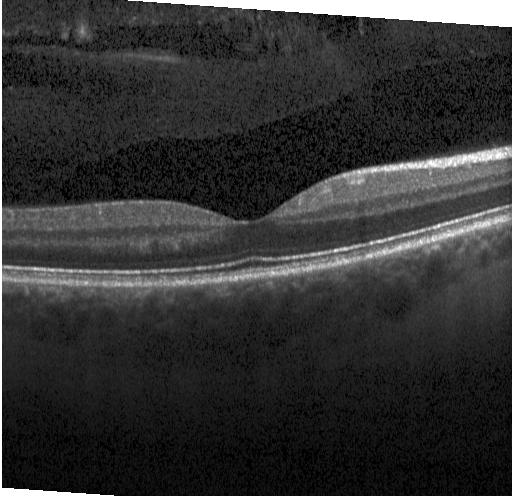
Spectral-domain optical coherence tomography, acquired on a Heidelberg Spectralis, OCT line scan — Macular OCT: no choroidal neovascularization, no diabetic macular edema, and no drusen.